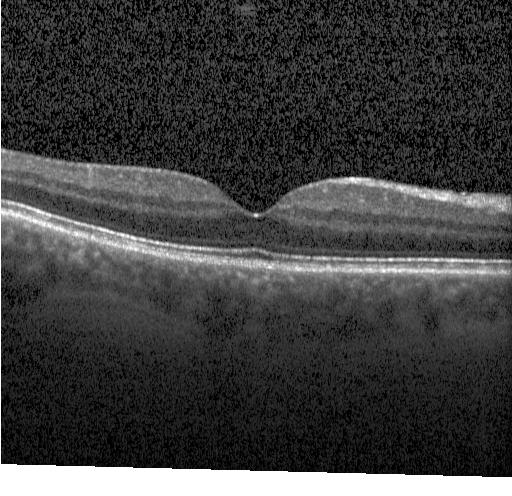

OCT finding: no evidence of choroidal neovascularization, diabetic macular edema, or drusen.